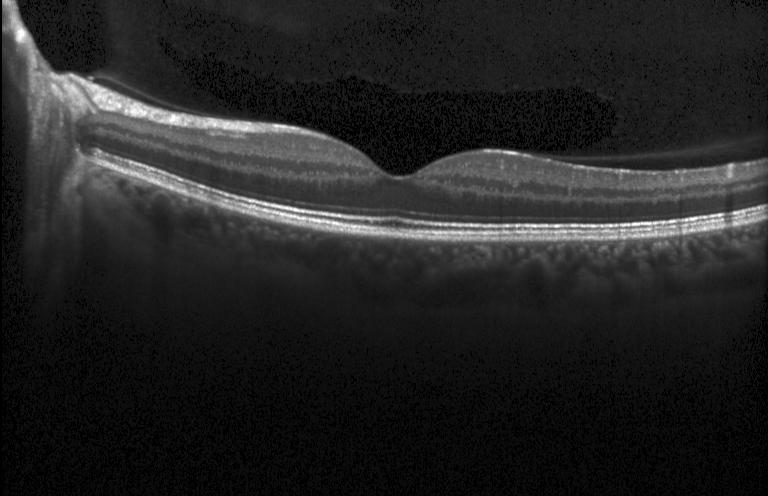 Optical coherence tomography scan. Spectral-domain optical coherence tomography. Heidelberg Spectralis. OCT finding: no evidence of choroidal neovascularization, diabetic macular edema, or drusen.